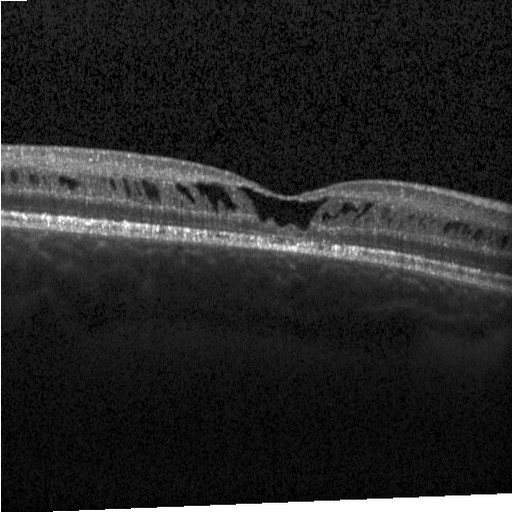

Retinal OCT cross-section. Spectral-domain optical coherence tomography — This B-scan demonstrates diabetic macular edema (DME).